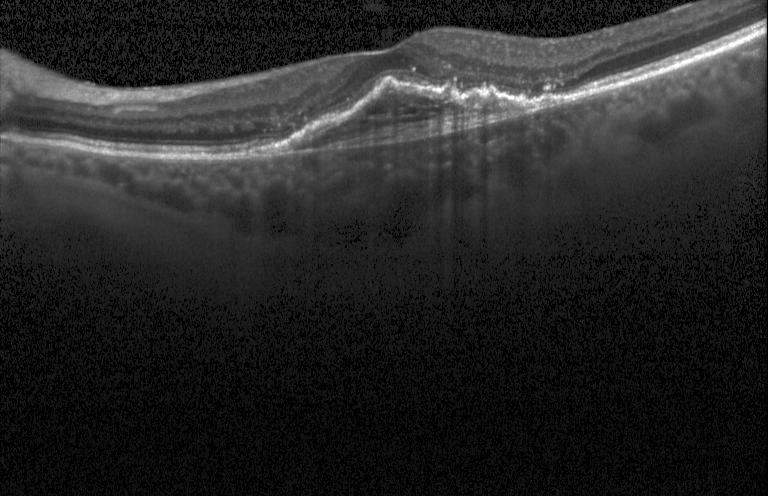
OCT B-scan showing a choroidal neovascular membrane.